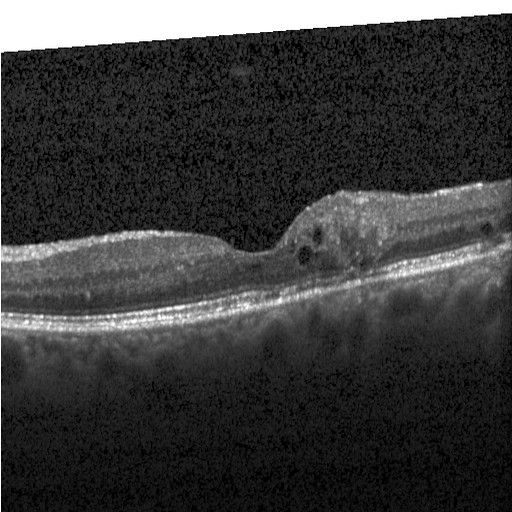
Heidelberg Spectralis, retinal OCT B-scan, centered on the fovea
Assessment: diabetic macular edema (DME).